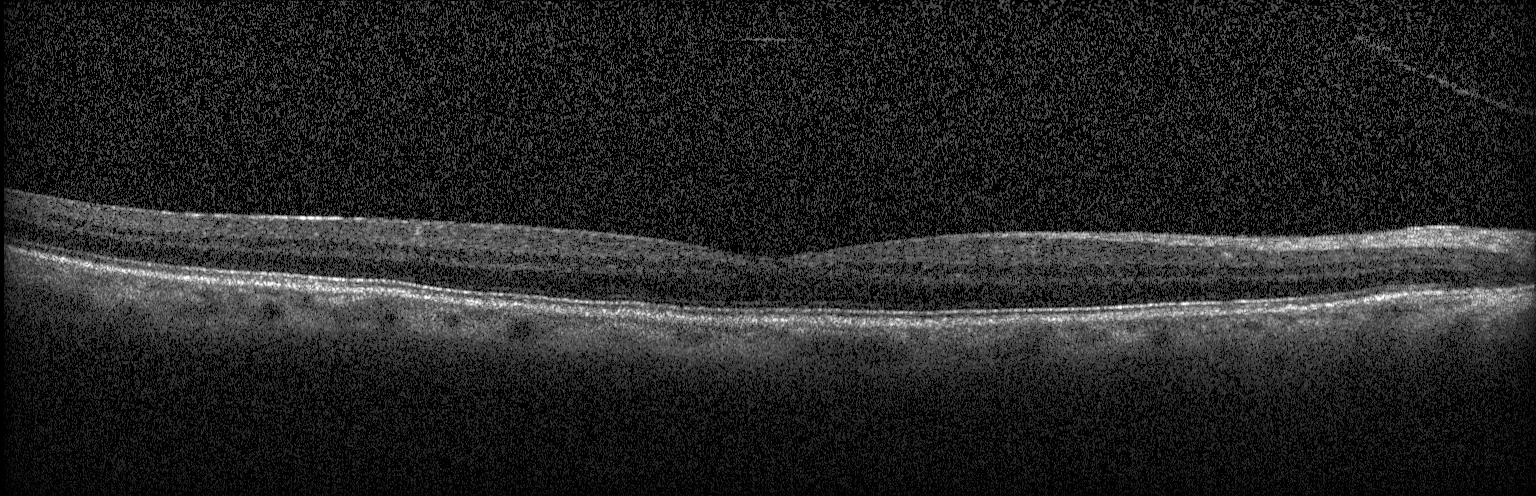

Retinal OCT B-scan — Diagnosis: no evidence of CNV, DME, or drusen.